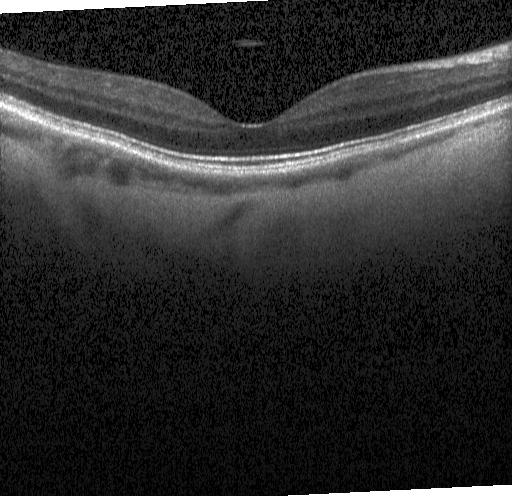
OCT scan showing no evidence of CNV, DME, or drusen.